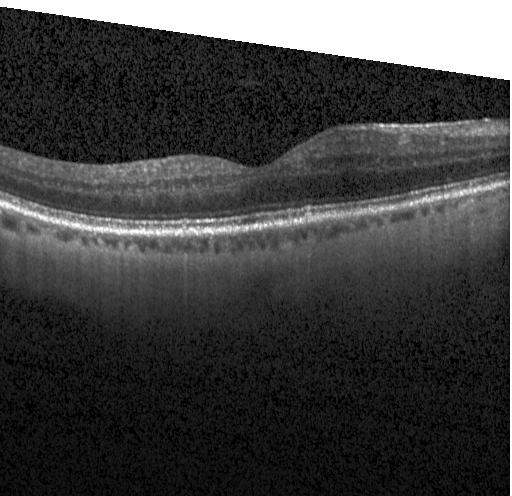 Heidelberg Spectralis, fovea-centered, OCT line scan, spectral-domain optical coherence tomography. Diagnosis: neither choroidal neovascularization, diabetic macular edema, nor drusen.